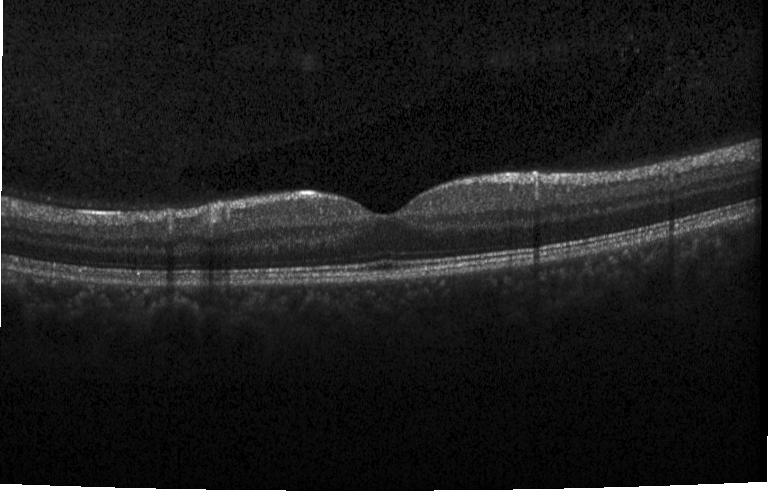 OCT B-scan
OCT finding: neither choroidal neovascularization, diabetic macular edema, nor drusen.